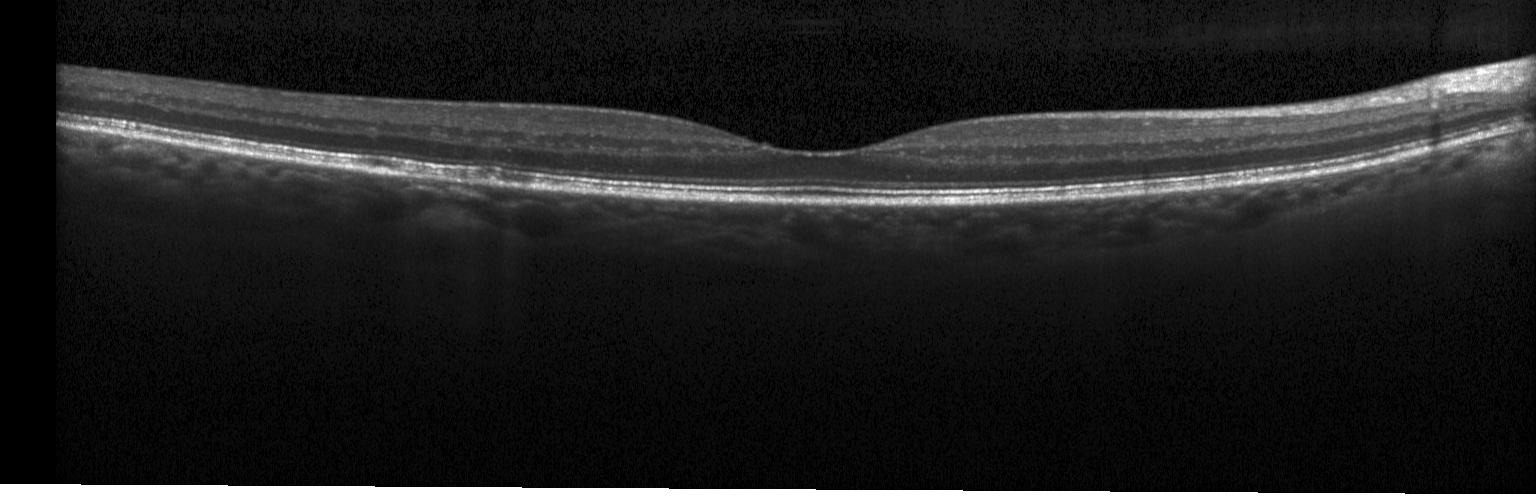 Macular OCT demonstrating neither choroidal neovascularization, diabetic macular edema, nor drusen.